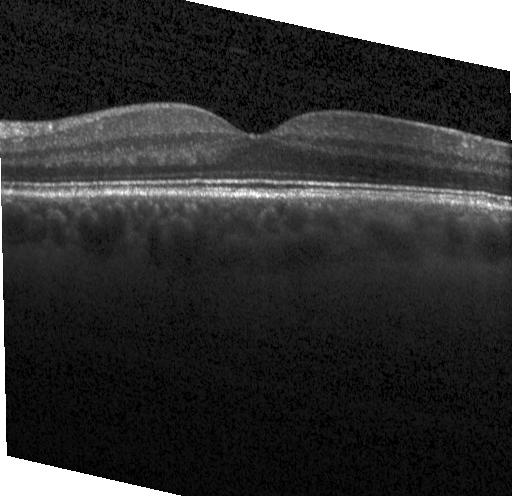
Diagnosis: no choroidal neovascularization, no diabetic macular edema, and no drusen.